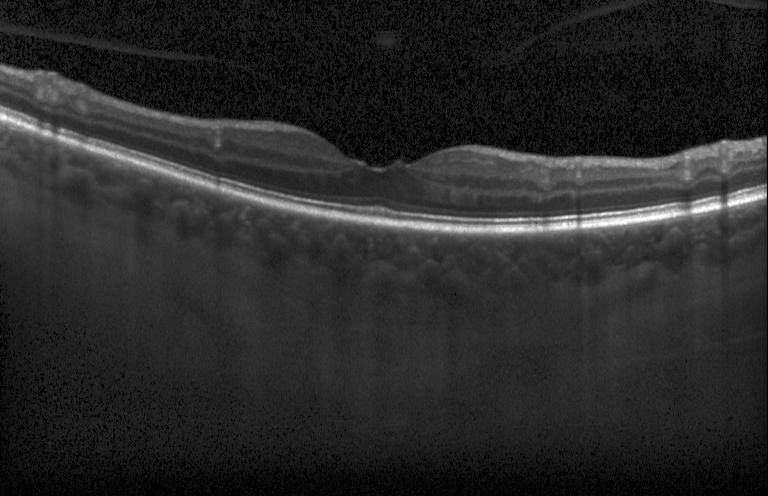 Retinal OCT cross-section showing no CNV, no DME, and no drusen.